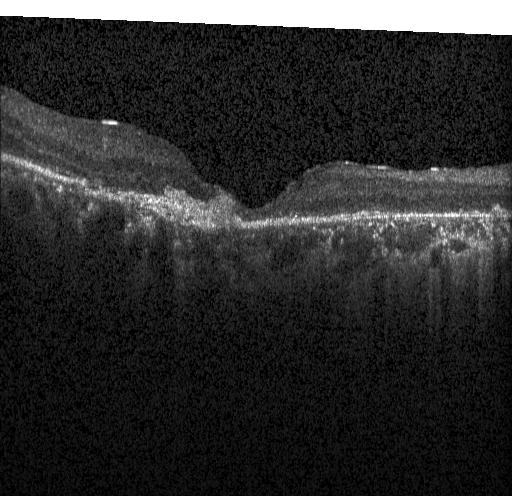

Spectral-domain optical coherence tomography. Retinal OCT cross-section
Dx: a choroidal neovascular membrane.